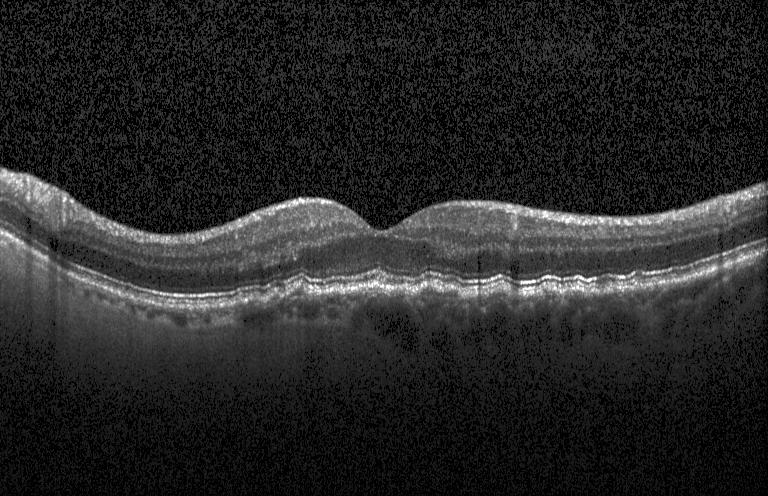

Impression: drusen.